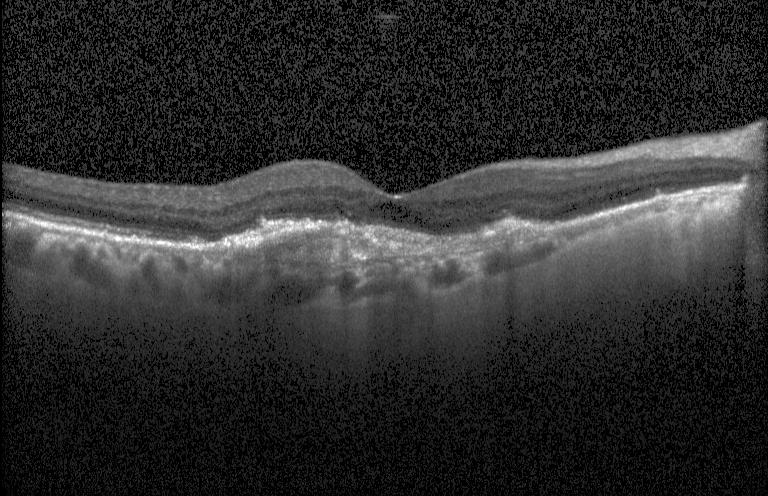 Spectral-domain optical coherence tomography; optical coherence tomography B-scan; instrument: Heidelberg Spectralis; fovea-centered
OCT finding: a choroidal neovascular membrane.